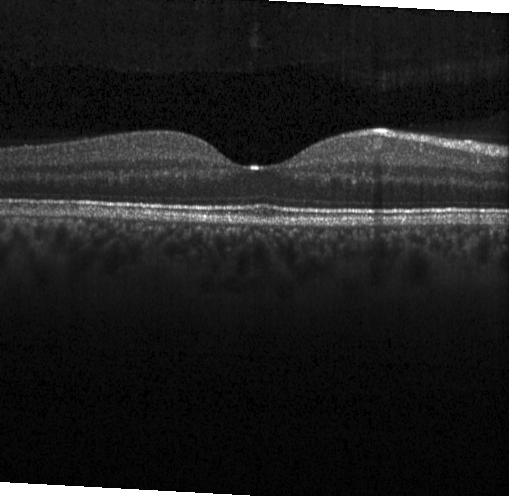
Spectral-domain OCT; macular scan; retinal OCT cross-section; Heidelberg Spectralis
This B-scan demonstrates no evidence of CNV, DME, or drusen.